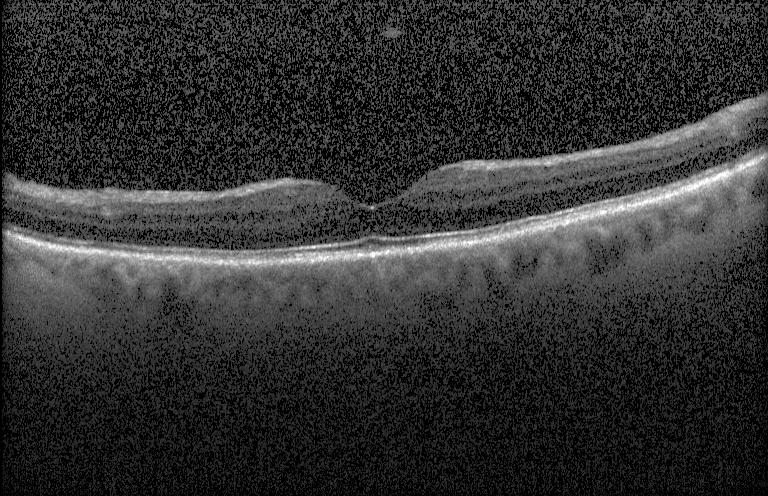

Optical coherence tomography scan. Impression: no evidence of choroidal neovascularization, diabetic macular edema, or drusen.